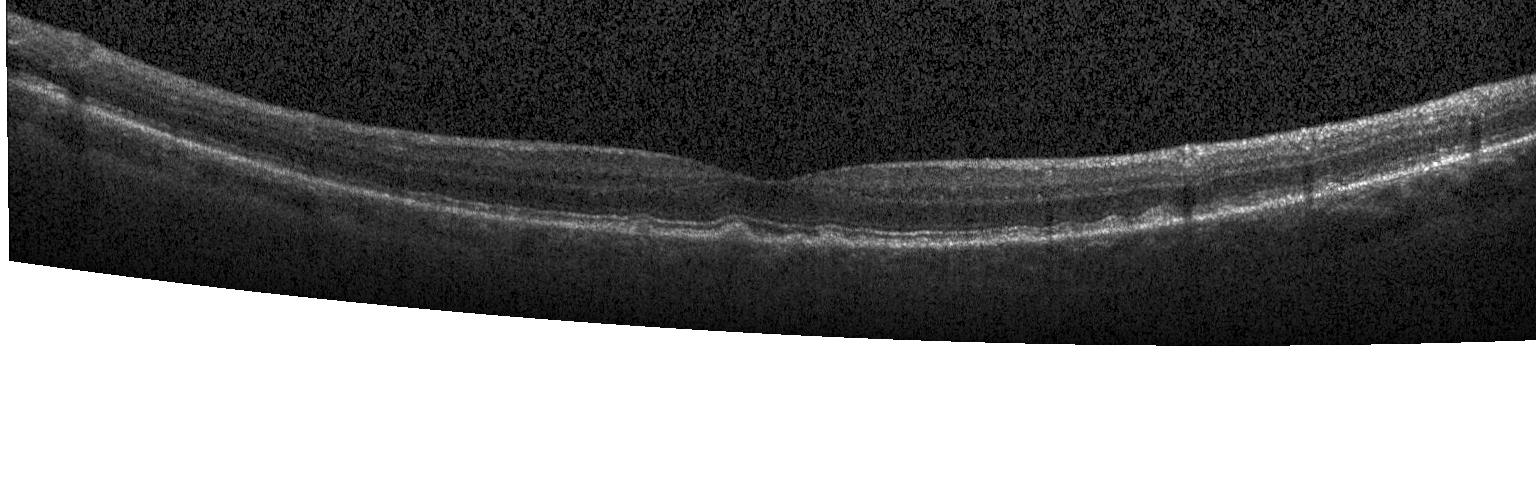
Dx: multiple drusen.